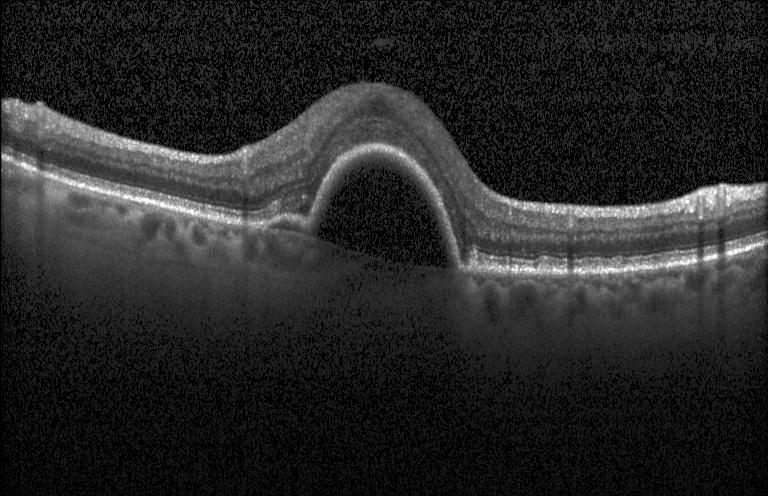 Impression: choroidal neovascularization (CNV).